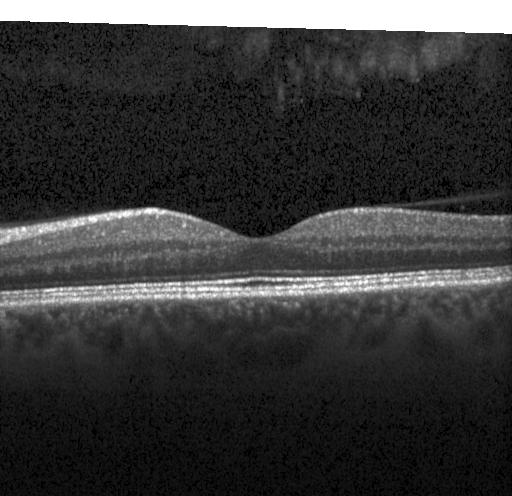

The scan shows no CNV, no DME, and no drusen.